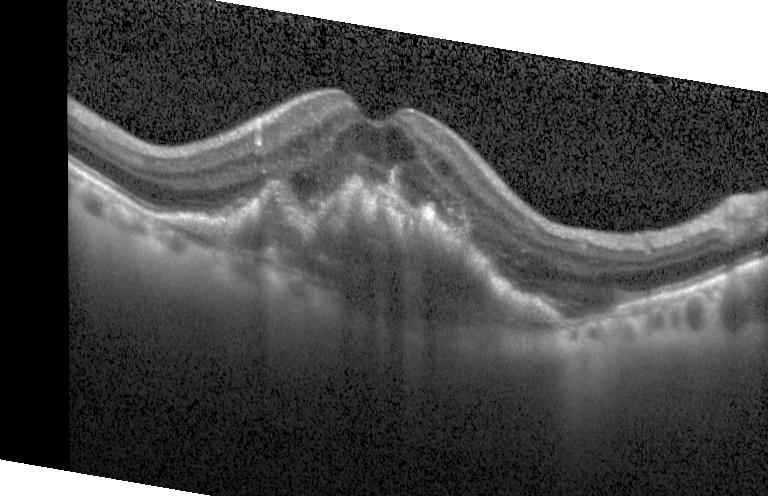

Fovea-centered · retinal OCT cross-section · acquired on a Heidelberg Spectralis
This B-scan demonstrates choroidal neovascularization.